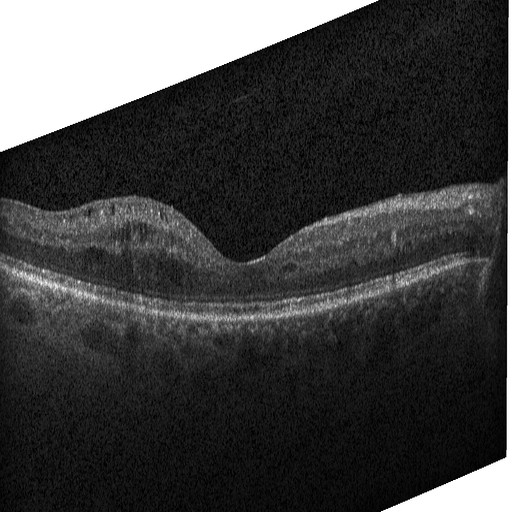 OCT finding: diabetic macular edema.